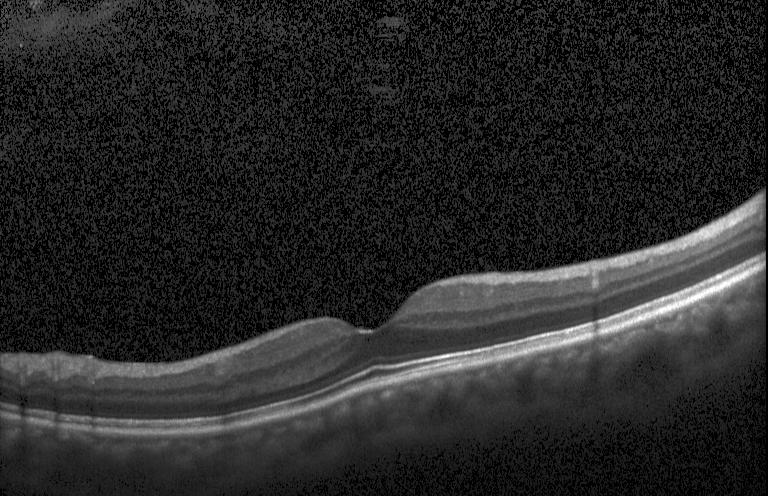 Diagnosis: no evidence of choroidal neovascularization, diabetic macular edema, or drusen.